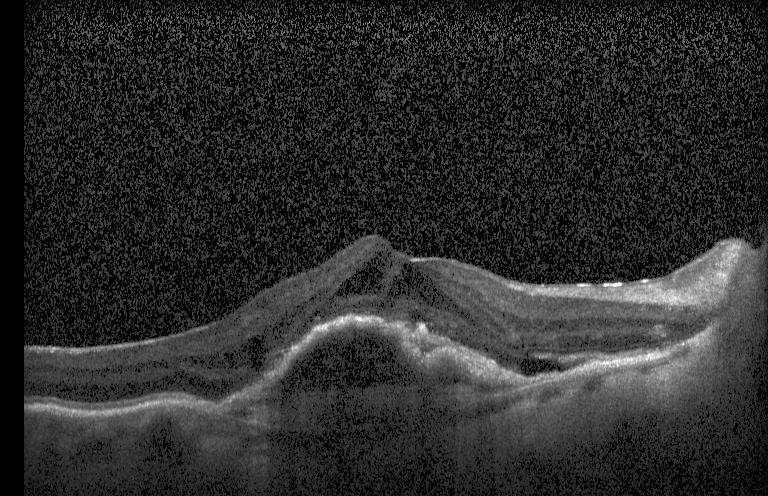 OCT line scan
A choroidal neovascular membrane.